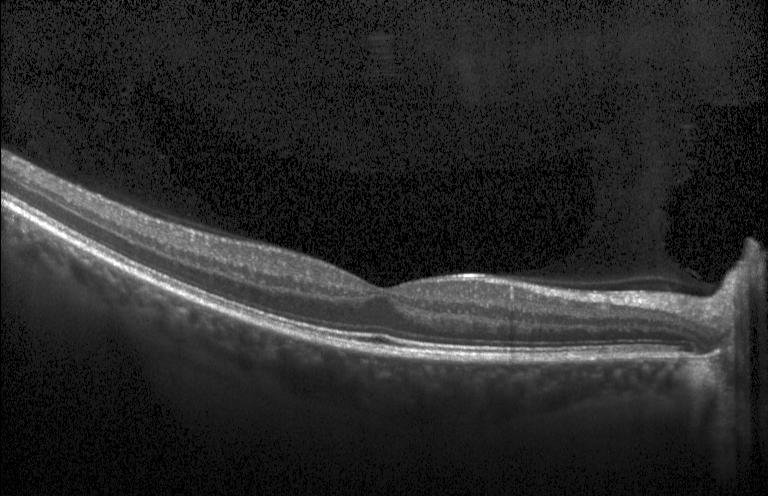

OCT line scan, SD-OCT. This B-scan demonstrates neither choroidal neovascularization, diabetic macular edema, nor drusen.